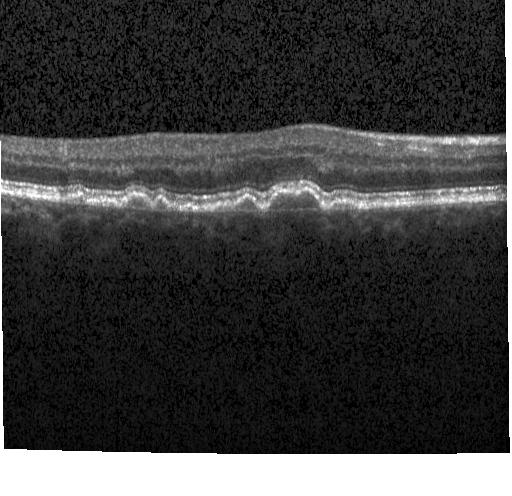

Optical coherence tomography B-scan, SD-OCT, centered on the fovea
Diagnosis: drusen.